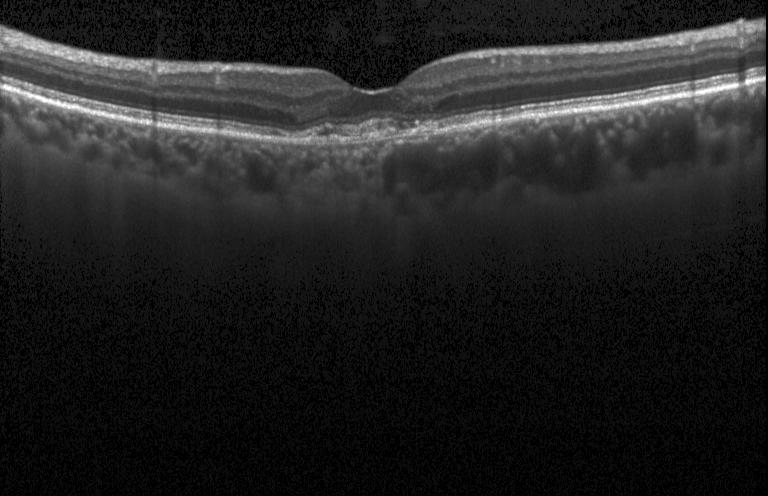

Spectral-domain optical coherence tomography. OCT line scan — Finding: choroidal neovascularization (CNV).